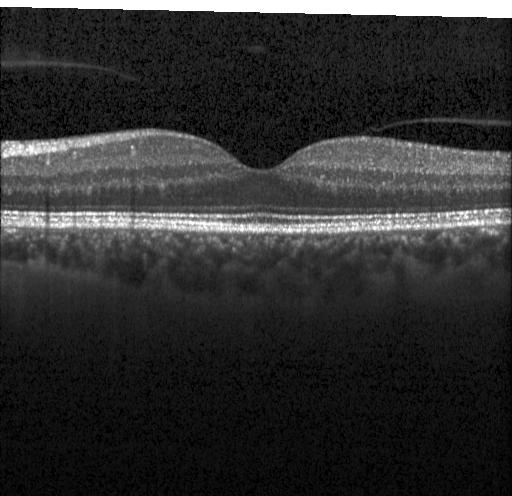
Impression: no evidence of choroidal neovascularization, diabetic macular edema, or drusen.